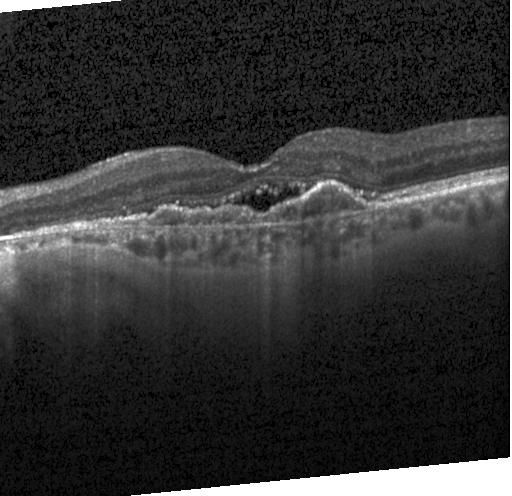 Optical coherence tomography scan, spectral-domain optical coherence tomography — Finding: choroidal neovascularization.